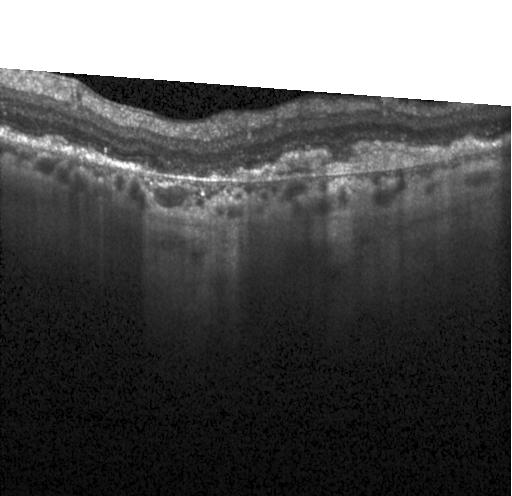
Acquired on a Heidelberg Spectralis. OCT line scan. Fovea-centered — Finding: a choroidal neovascular membrane.